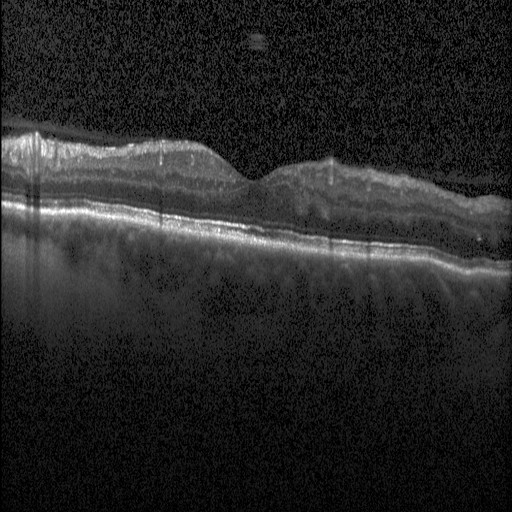 Spectral-domain optical coherence tomography; macular scan; instrument: Heidelberg Spectralis; OCT line scan — Macular OCT: diabetic macular edema (DME).